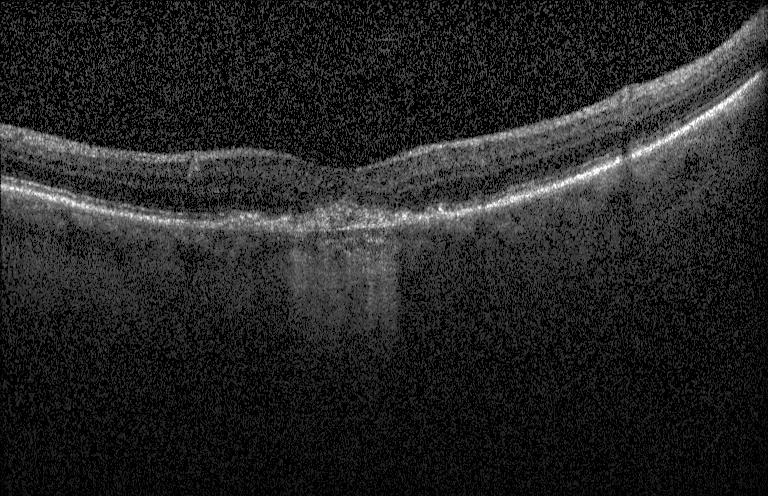
Retinal OCT B-scan; Heidelberg Spectralis OCT system.
Dx: a choroidal neovascular membrane.